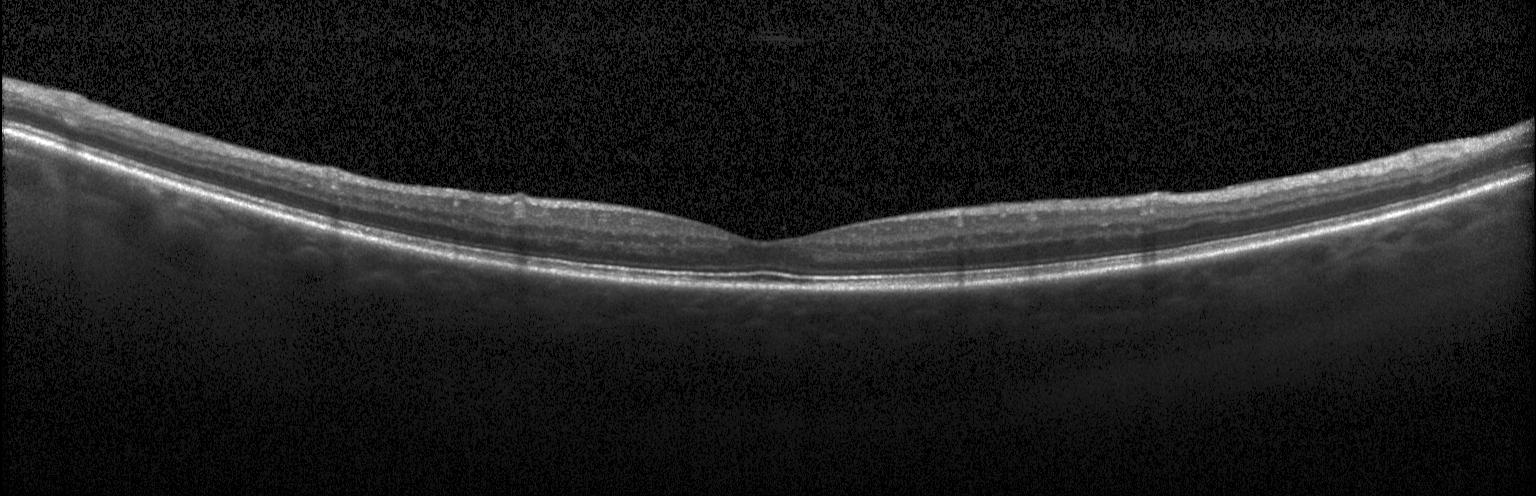
Macular scan, optical coherence tomography B-scan. Dx: no CNV, DME, or drusen.